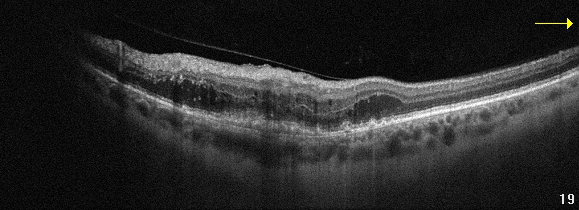 Retinal OCT cross-section · through the macula
Finding: AMD.